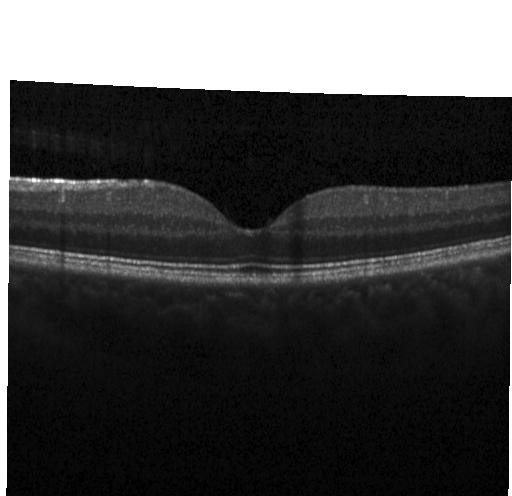
Retinal OCT cross-section, through the macula
Macular OCT: no choroidal neovascularization, no diabetic macular edema, and no drusen.